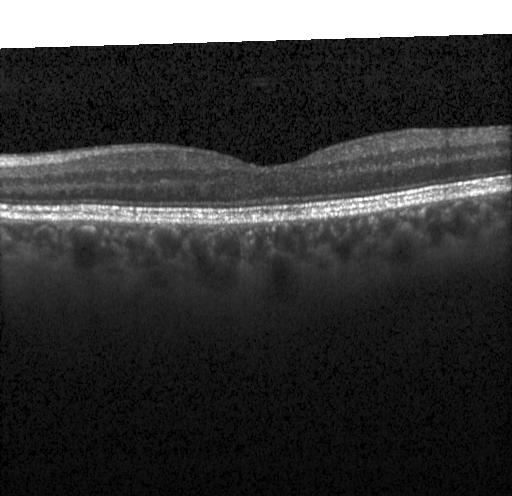
OCT B-scan showing no CNV, DME, or drusen.